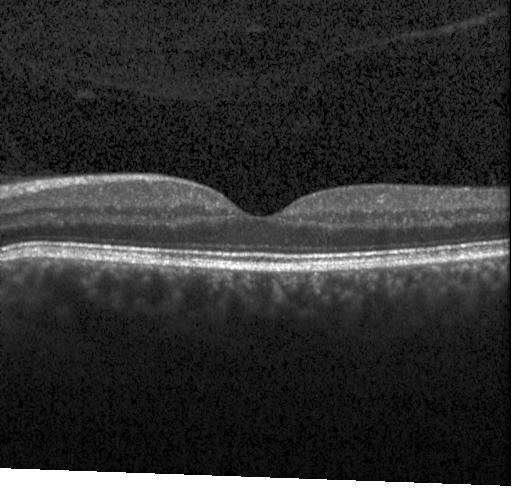
Acquired on a Heidelberg Spectralis; retinal OCT B-scan; centered on the fovea — Neither choroidal neovascularization, diabetic macular edema, nor drusen.